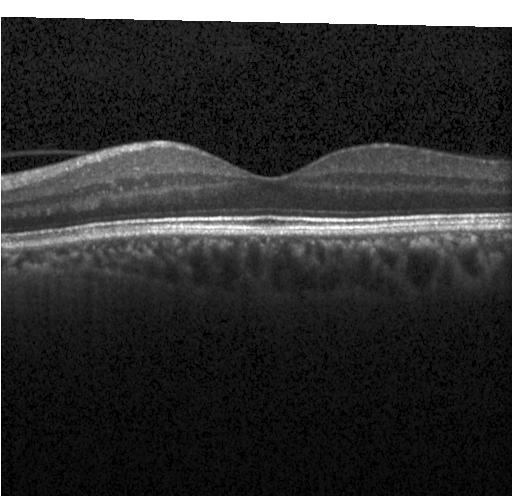
Macular OCT demonstrating no evidence of choroidal neovascularization, diabetic macular edema, or drusen.